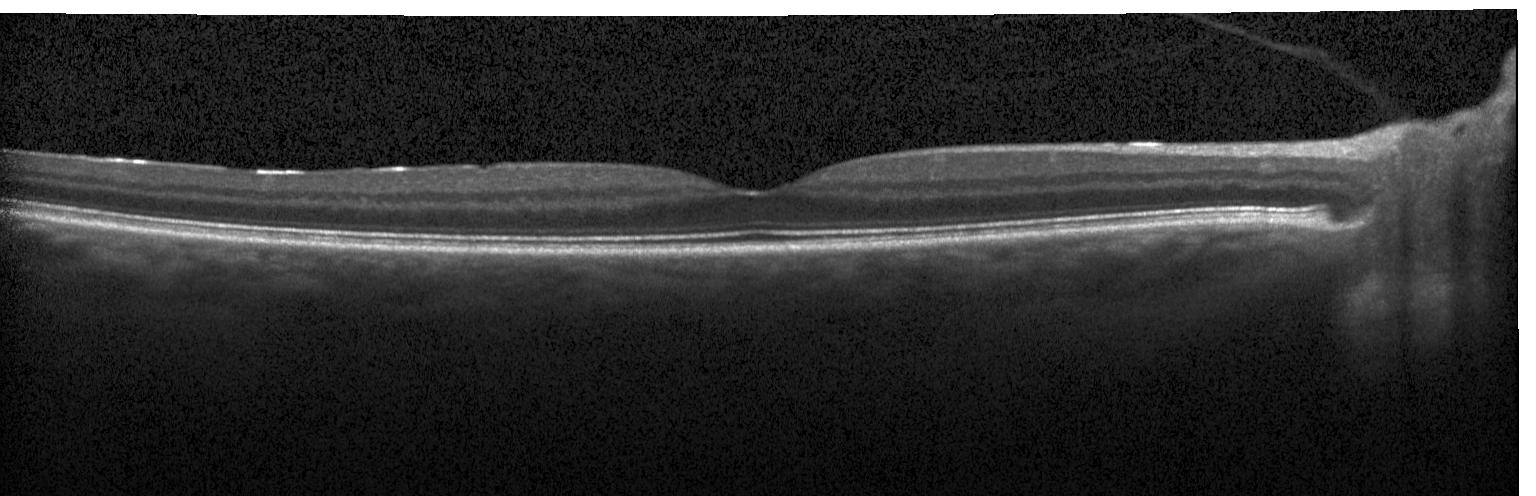
OCT finding: neither CNV, DME, nor drusen.